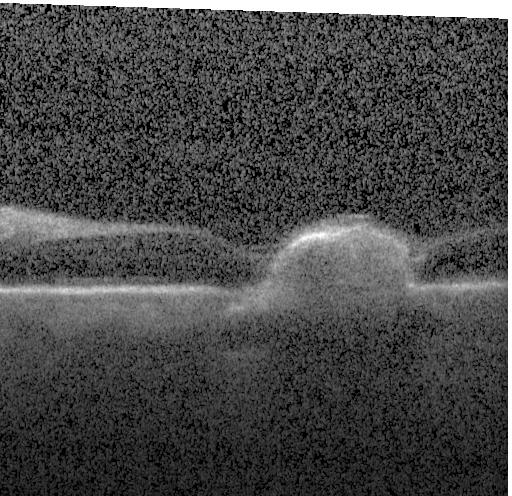

Optical coherence tomography scan; instrument: Heidelberg Spectralis; through the macula. This B-scan demonstrates CNV.